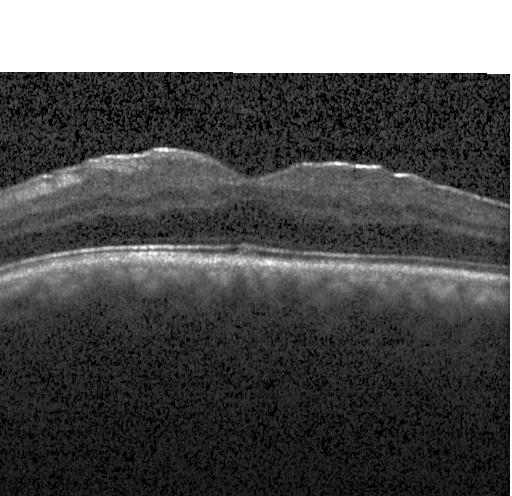 Optical coherence tomography B-scan. Dx: neither choroidal neovascularization, diabetic macular edema, nor drusen.